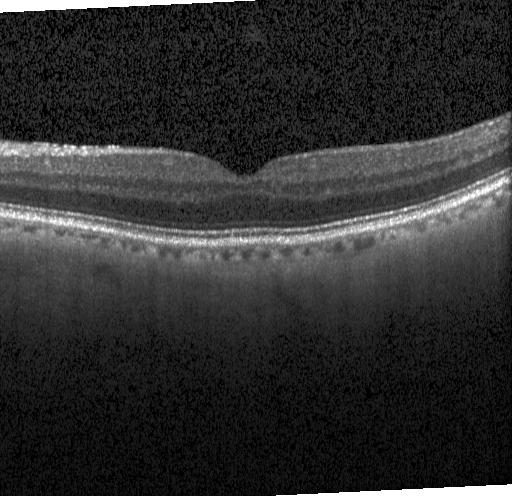
The scan shows no choroidal neovascularization, diabetic macular edema, or drusen.